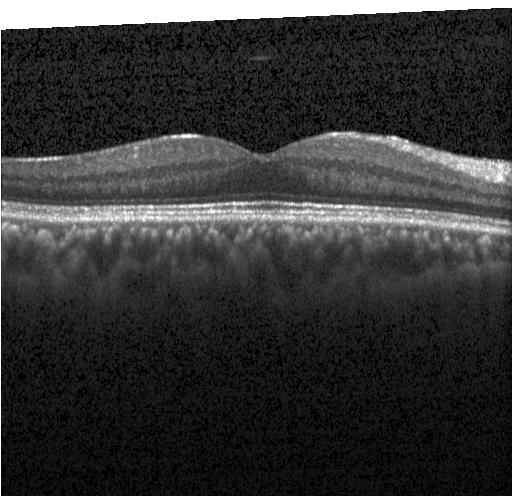 Spectral-domain OCT B-scan: no evidence of choroidal neovascularization, diabetic macular edema, or drusen.